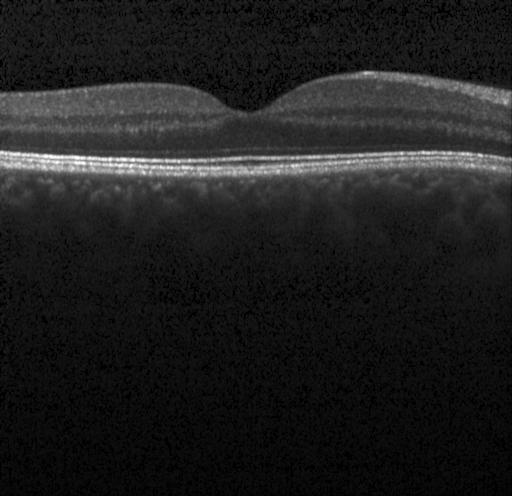
OCT B-scan showing no choroidal neovascularization, diabetic macular edema, or drusen.